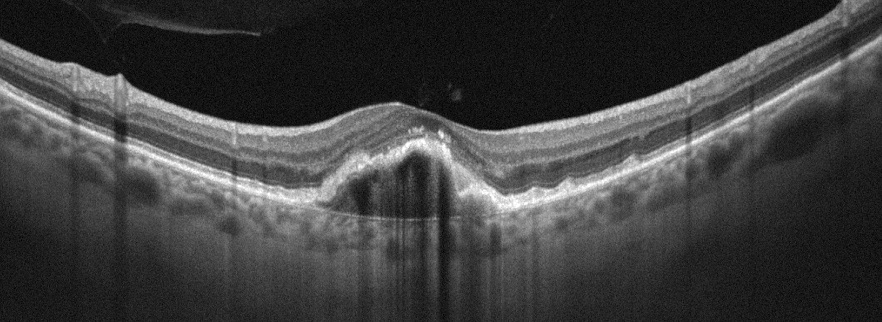
OCT B-scan; through the macula; instrument: Optovue Avanti RTVue XR — Age-related macular degeneration.